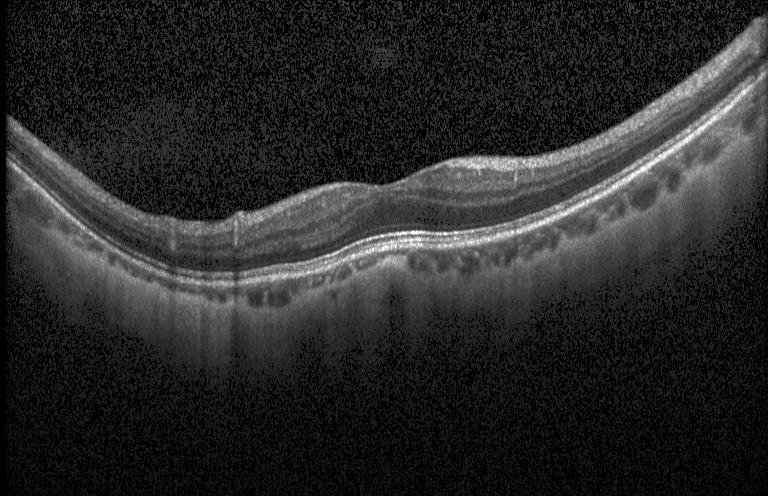
Diagnosis: no evidence of CNV, DME, or drusen.